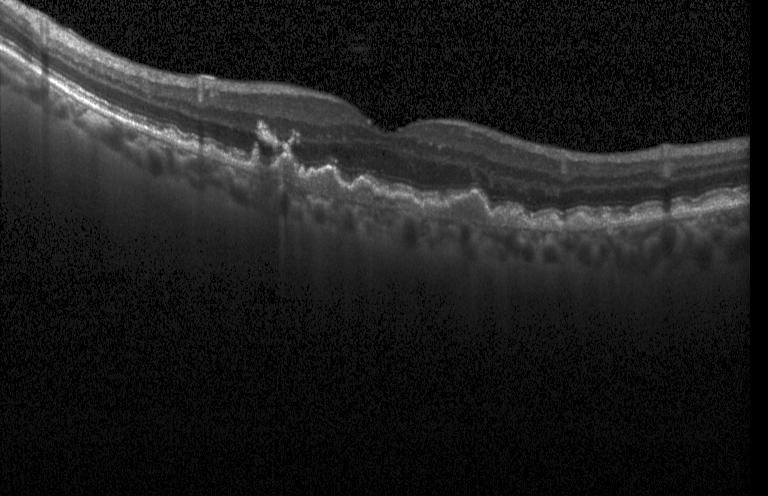
The scan shows a choroidal neovascular membrane.